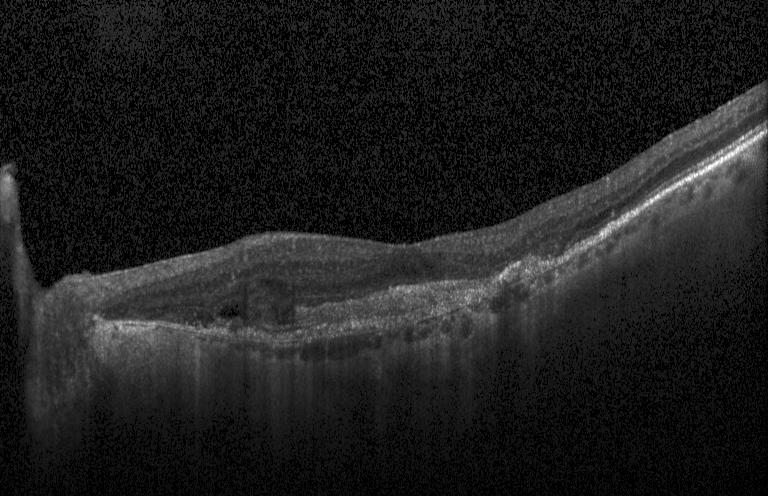

Impression: choroidal neovascularization.